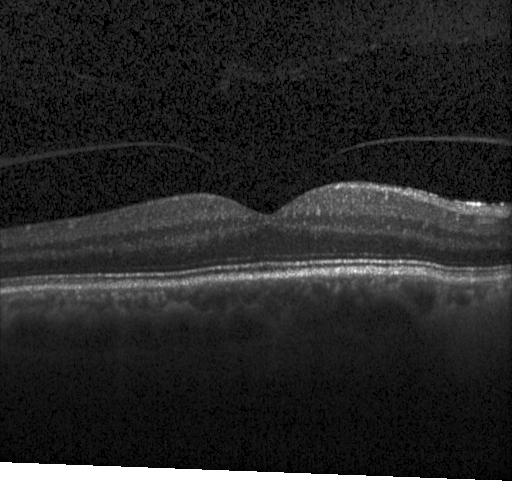 SD-OCT. Centered on the fovea. Optical coherence tomography scan. Acquired on a Heidelberg Spectralis.
Assessment: no choroidal neovascularization, diabetic macular edema, or drusen.